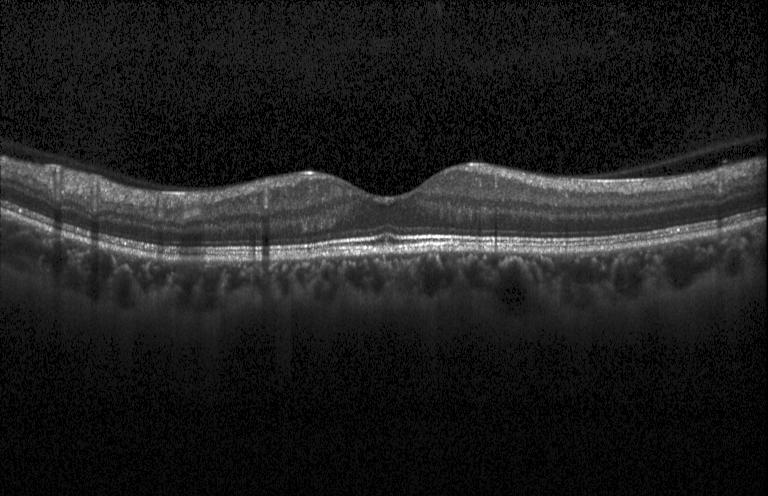 OCT line scan
Impression: no choroidal neovascularization, diabetic macular edema, or drusen.